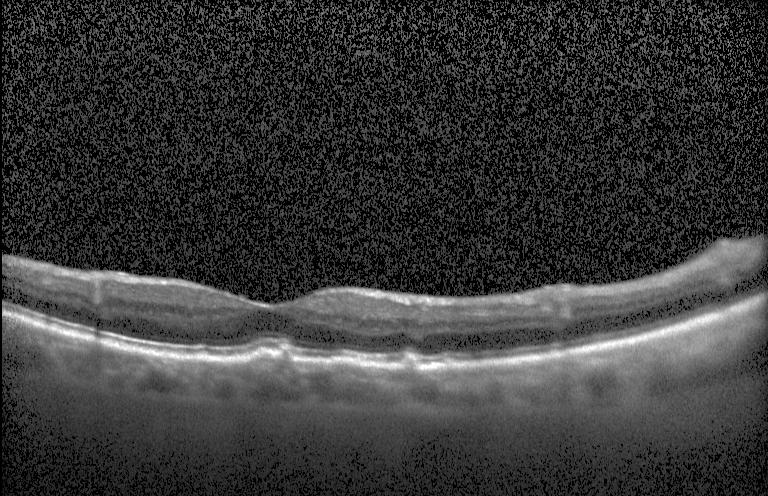

This B-scan demonstrates sub-RPE drusenoid deposits.